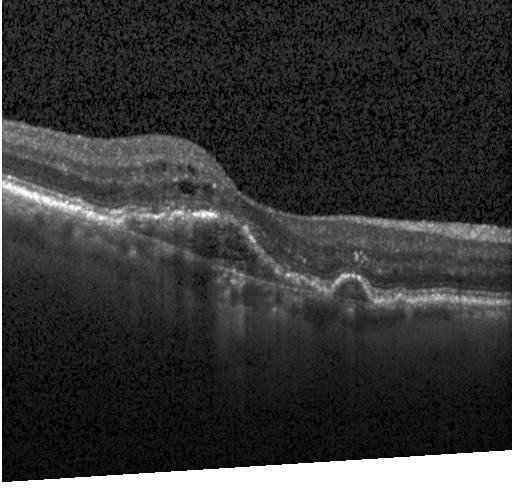

Macular OCT: a choroidal neovascular membrane.